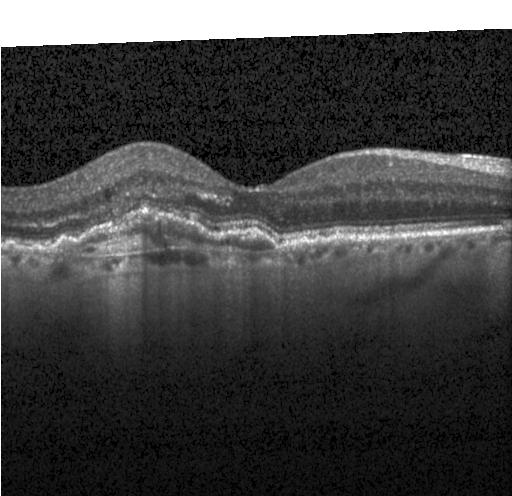

Spectral-domain optical coherence tomography, horizontal scan through the fovea, instrument: Heidelberg Spectralis, optical coherence tomography scan
Finding: choroidal neovascularization (CNV).